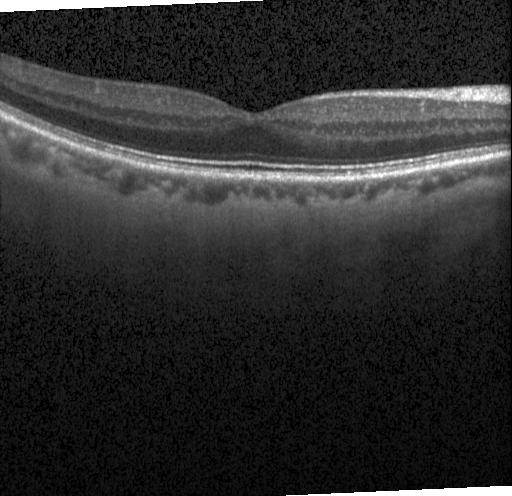
This B-scan demonstrates no choroidal neovascularization, no diabetic macular edema, and no drusen.